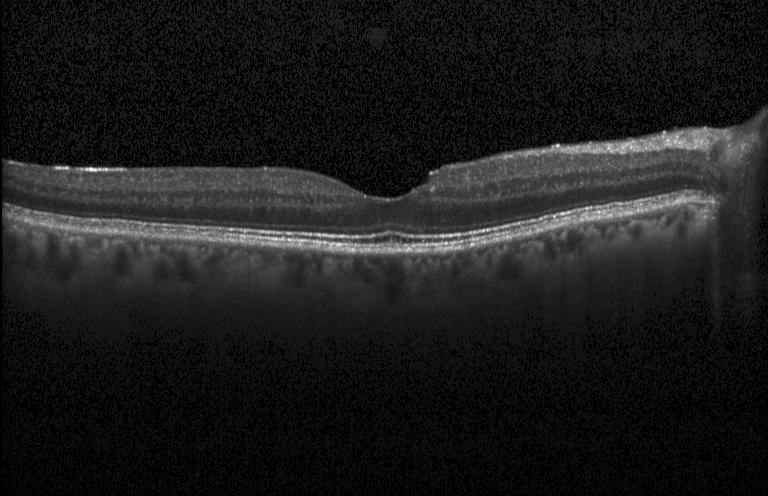
Heidelberg Spectralis OCT system. Macular scan. OCT line scan — Diagnosis: no CNV, no DME, and no drusen.